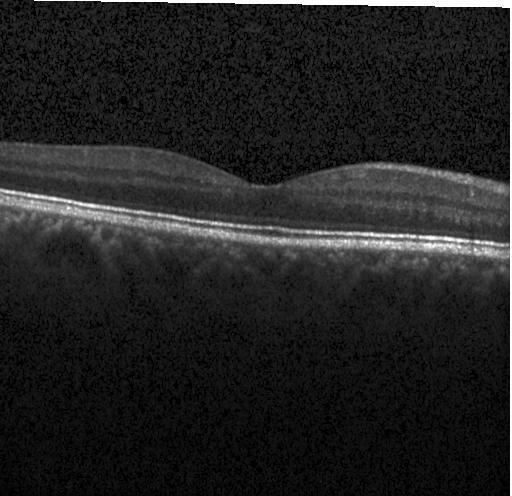

Optical coherence tomography B-scan; SD-OCT; Heidelberg Spectralis
Dx: no evidence of CNV, DME, or drusen.